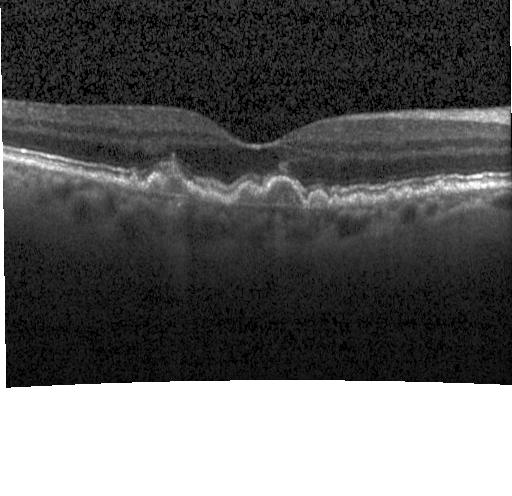 Retinal OCT cross-section. Macular OCT: multiple drusen.